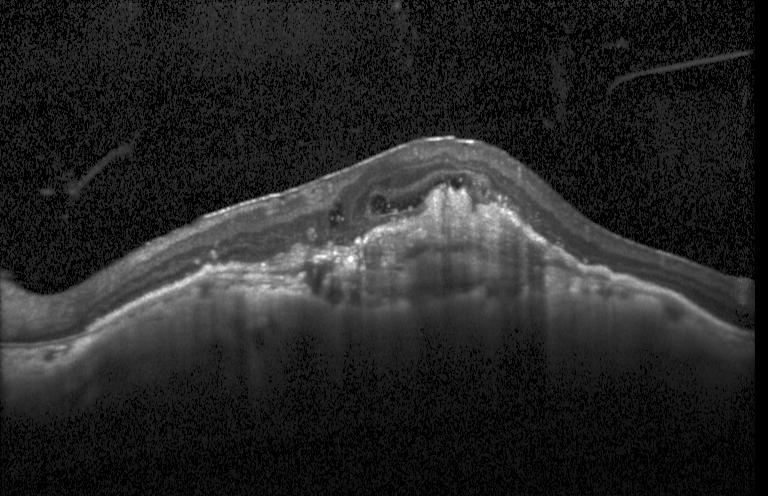
Through the macula; spectral-domain optical coherence tomography; acquired on a Heidelberg Spectralis; optical coherence tomography B-scan
Assessment: choroidal neovascularization.